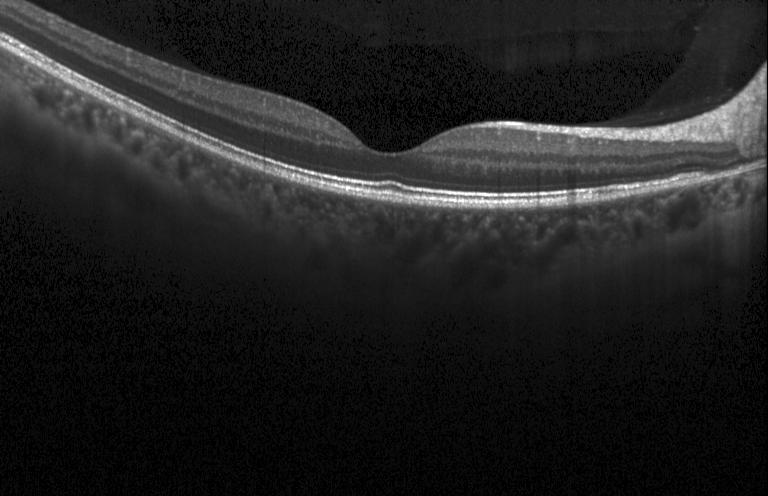
Through the macula · retinal OCT cross-section
Finding: neither choroidal neovascularization, diabetic macular edema, nor drusen.